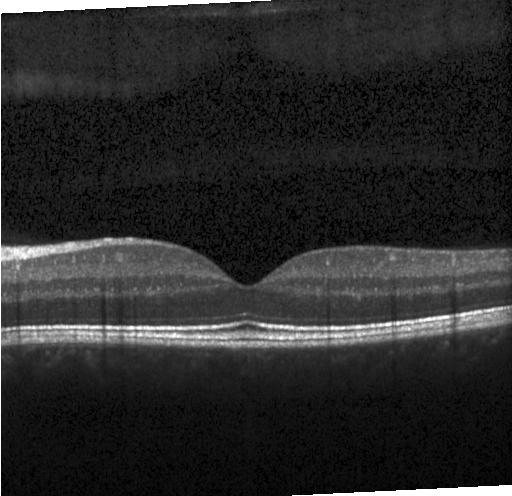
Spectral-domain optical coherence tomography, through the macula, Heidelberg Spectralis OCT system, optical coherence tomography B-scan — The scan shows no CNV, no DME, and no drusen.